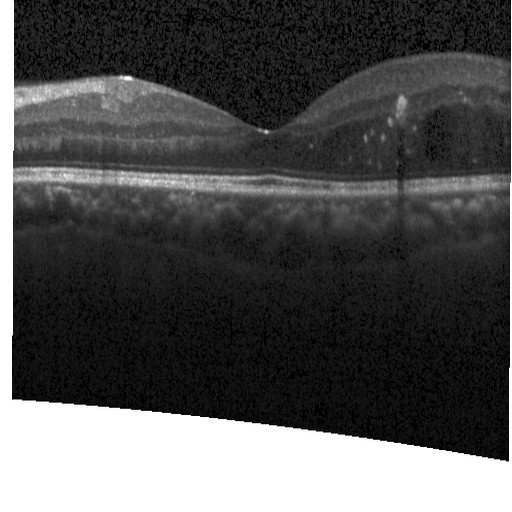 Spectral-domain optical coherence tomography; optical coherence tomography B-scan. Dx: diabetic macular edema (DME).